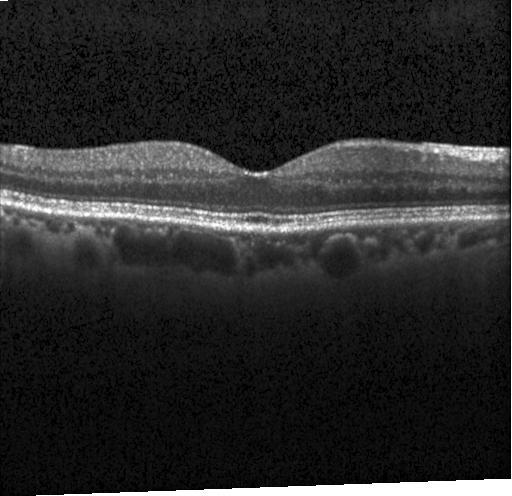
Assessment: neither choroidal neovascularization, diabetic macular edema, nor drusen.